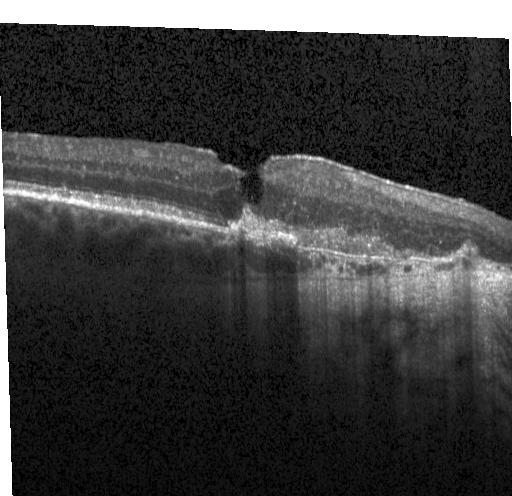
Acquired on a Heidelberg Spectralis. Optical coherence tomography scan — Diagnosis: a choroidal neovascular membrane.